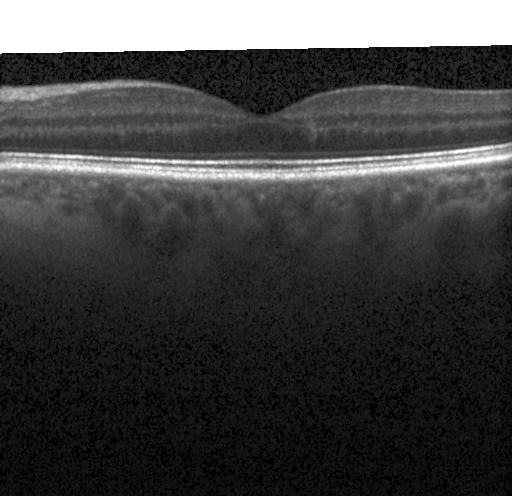

OCT line scan, through the macula, spectral-domain OCT, instrument: Heidelberg Spectralis — Dx: no evidence of choroidal neovascularization, diabetic macular edema, or drusen.